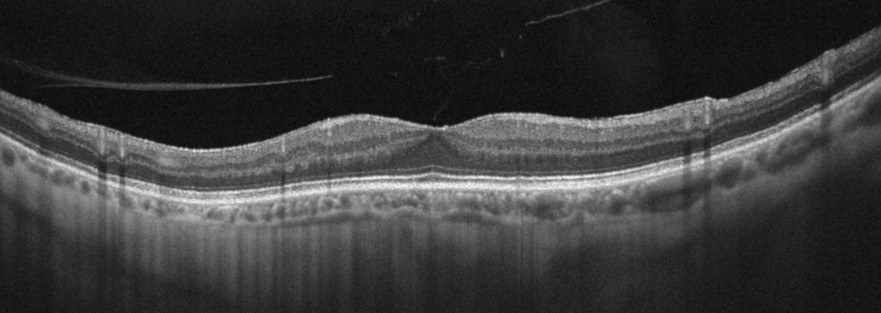 Optovue Avanti RTVue XR. Retinal OCT B-scan
Macular OCT: absence of AMD, DME, ERM, RAO, RVO, and vitreomacular interface disease.